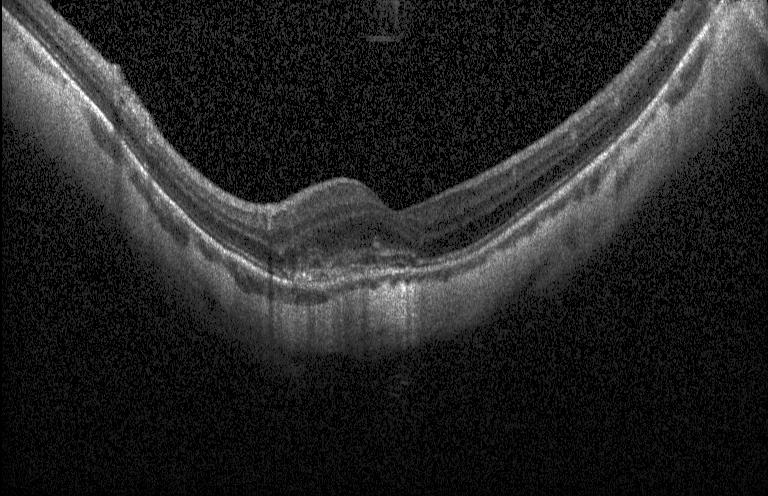

OCT B-scan; fovea-centered; spectral-domain optical coherence tomography; Heidelberg Spectralis.
Impression: choroidal neovascularization (CNV).